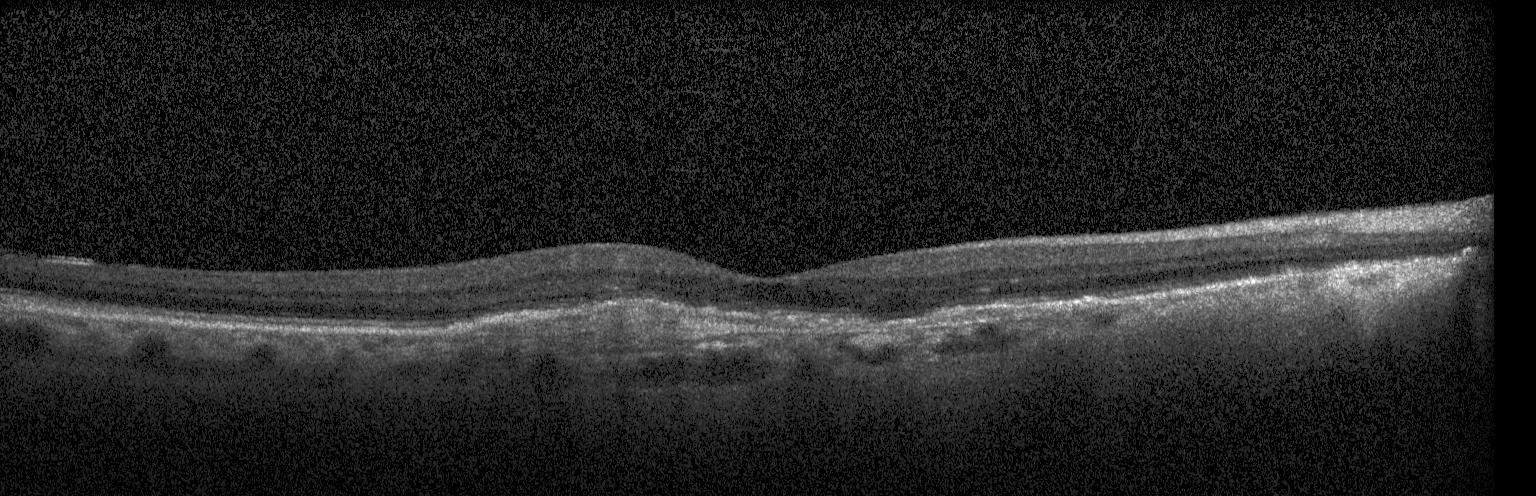 Spectral-domain OCT B-scan: a choroidal neovascular membrane.